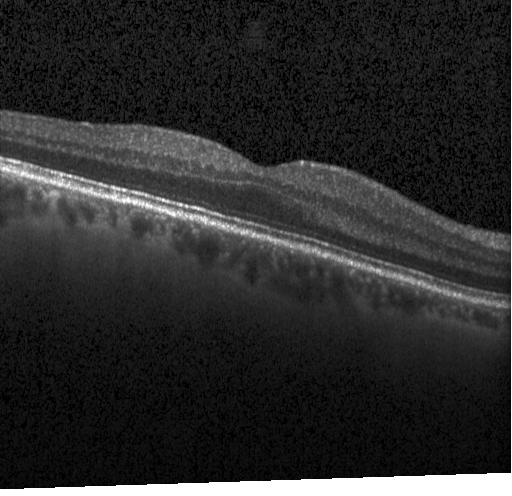
Centered on the fovea. Optical coherence tomography scan. Spectral-domain OCT. Acquired on a Heidelberg Spectralis — Finding: no choroidal neovascularization, no diabetic macular edema, and no drusen.